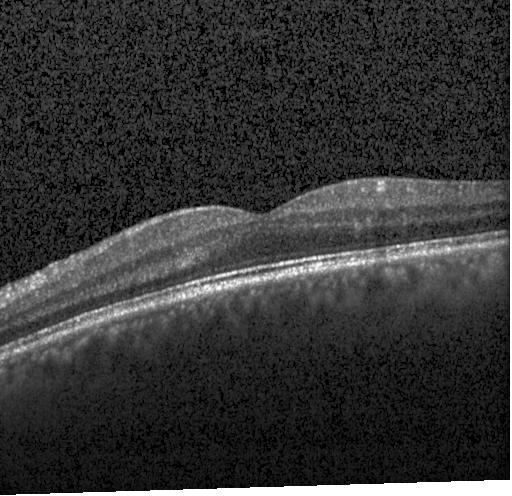 SD-OCT. Through the macula. Retinal OCT cross-section.
Impression: no evidence of CNV, DME, or drusen.